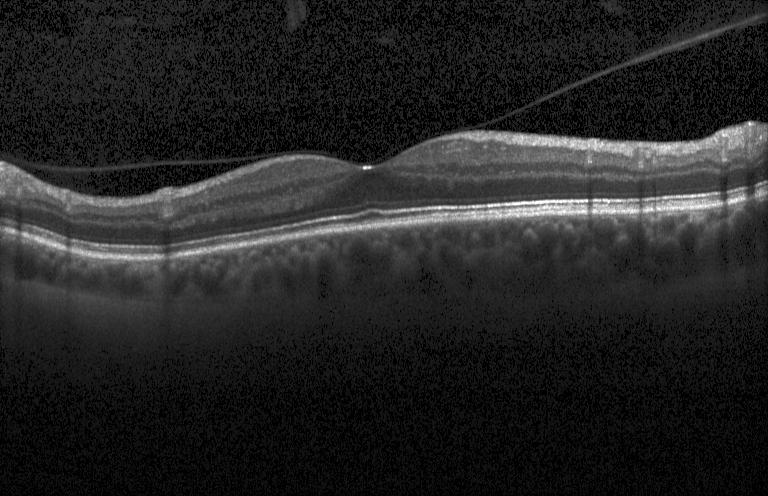
OCT B-scan showing neither CNV, DME, nor drusen.